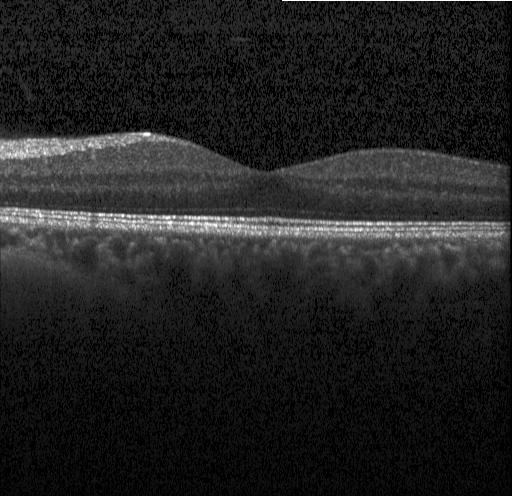

Spectral-domain OCT B-scan: no choroidal neovascularization, no diabetic macular edema, and no drusen.